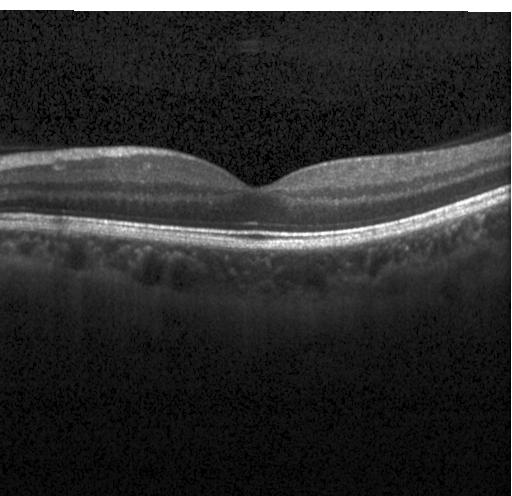 Instrument: Heidelberg Spectralis. Retinal OCT B-scan. Through the macula.
Assessment: no choroidal neovascularization, no diabetic macular edema, and no drusen.